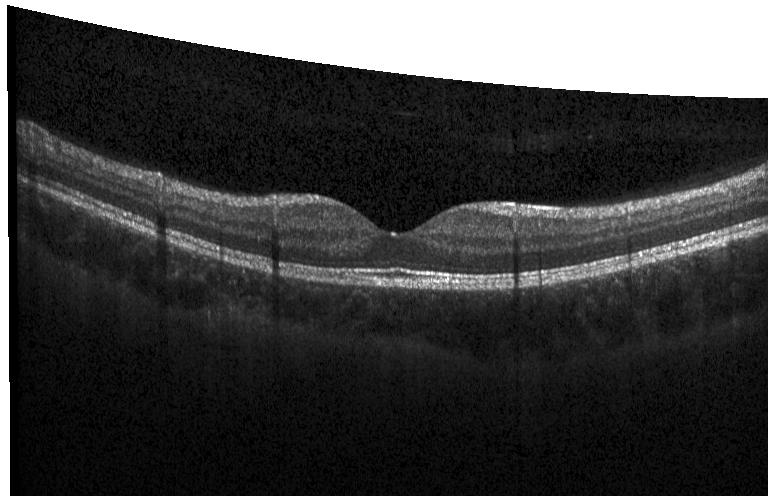 Spectral-domain optical coherence tomography · instrument: Heidelberg Spectralis · retinal OCT cross-section. Finding: no choroidal neovascularization, diabetic macular edema, or drusen.